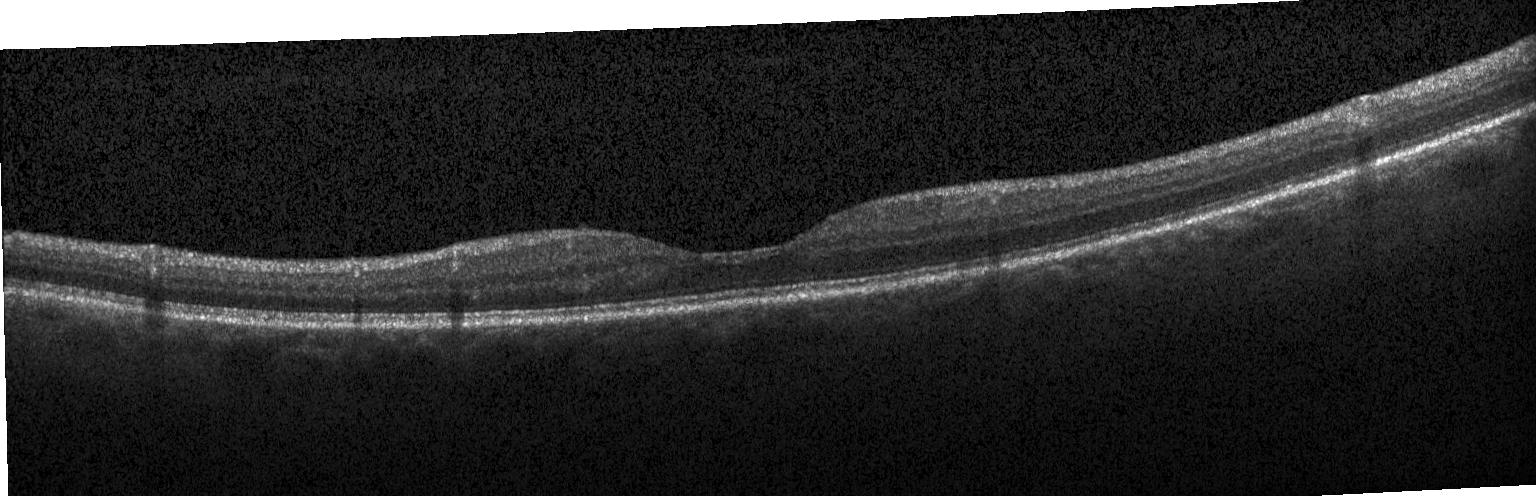
The scan shows no evidence of CNV, DME, or drusen.